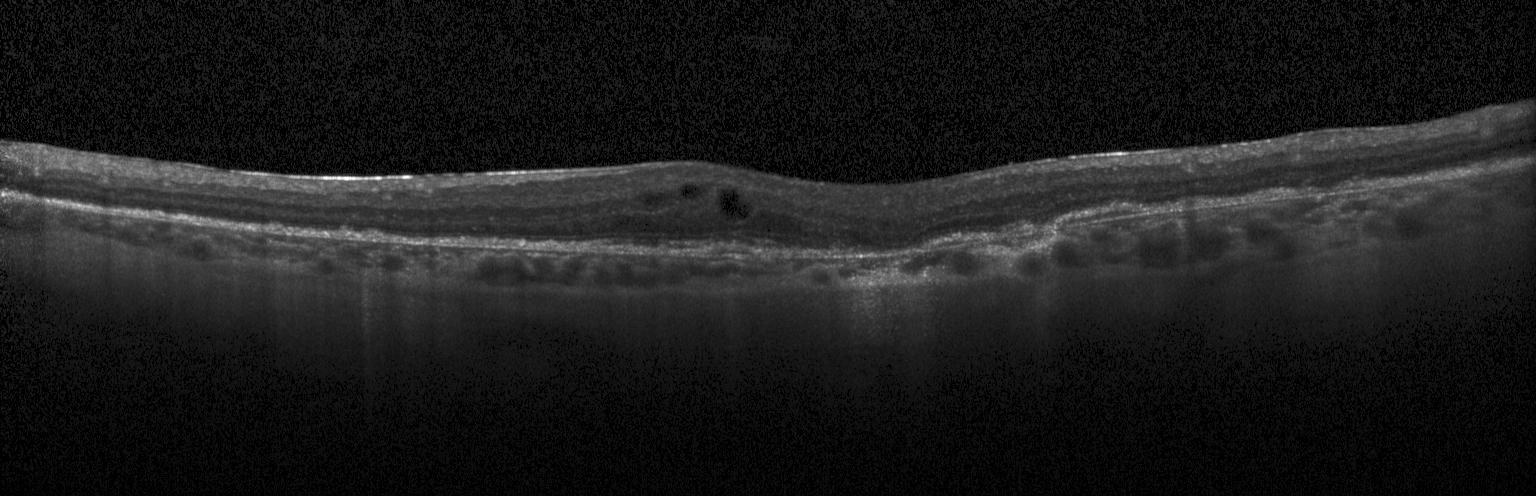 OCT finding: a choroidal neovascular membrane.